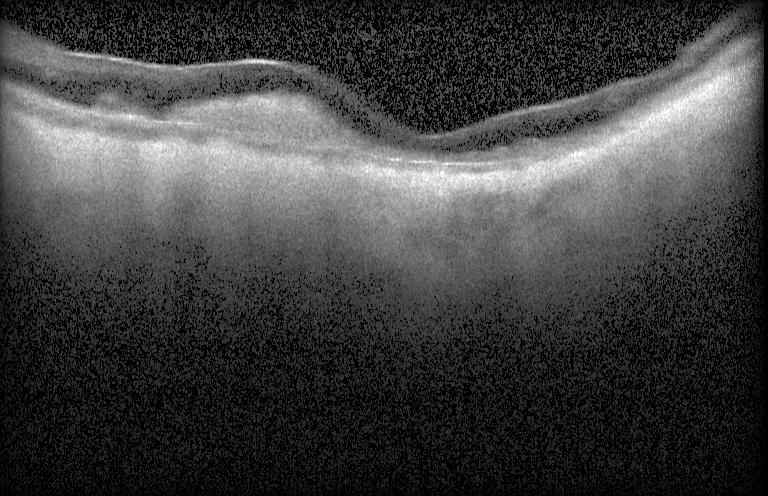

Spectral-domain OCT B-scan: a choroidal neovascular membrane.